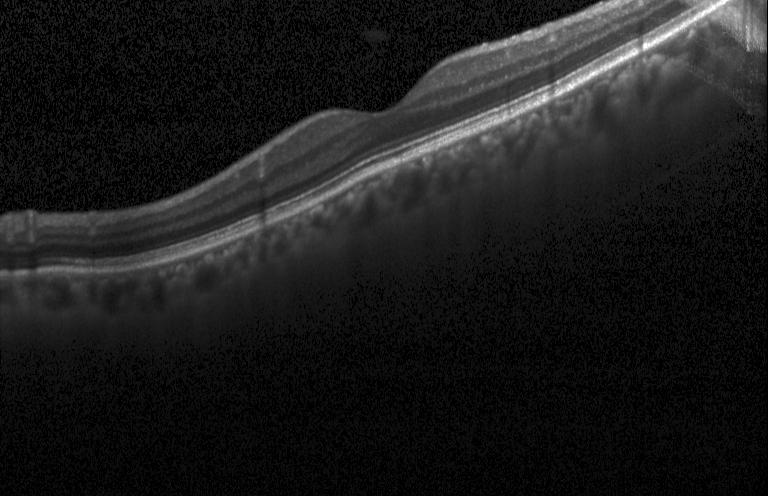
OCT line scan
Dx: neither choroidal neovascularization, diabetic macular edema, nor drusen.